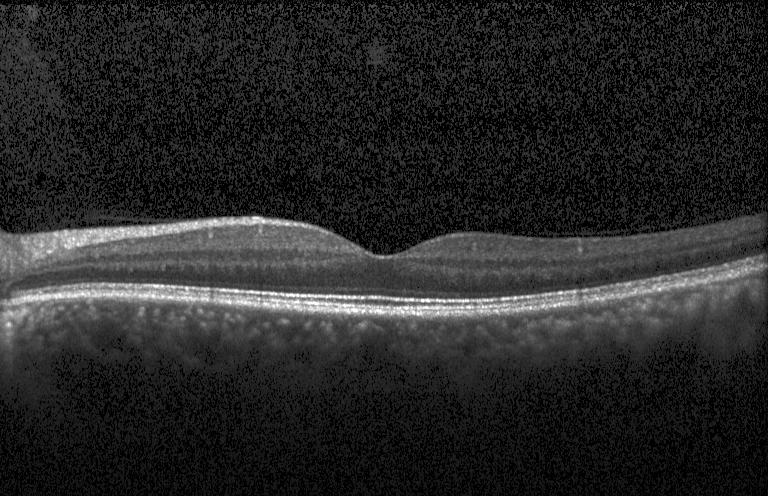

OCT finding: no choroidal neovascularization, no diabetic macular edema, and no drusen.